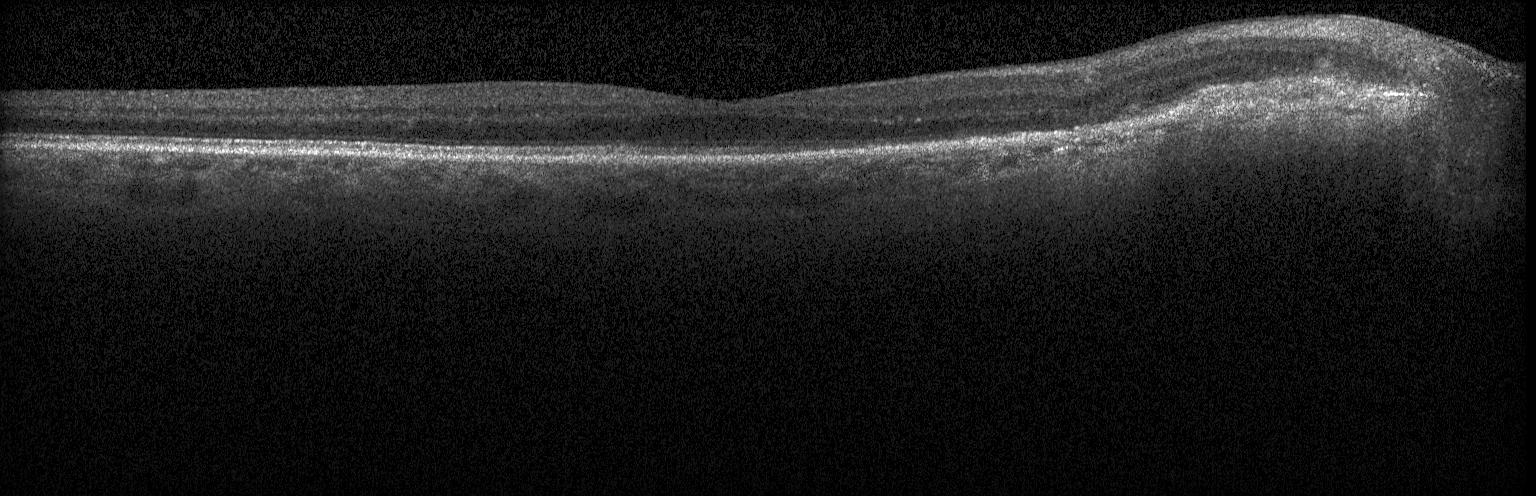 OCT line scan · Heidelberg Spectralis OCT system. A choroidal neovascular membrane.